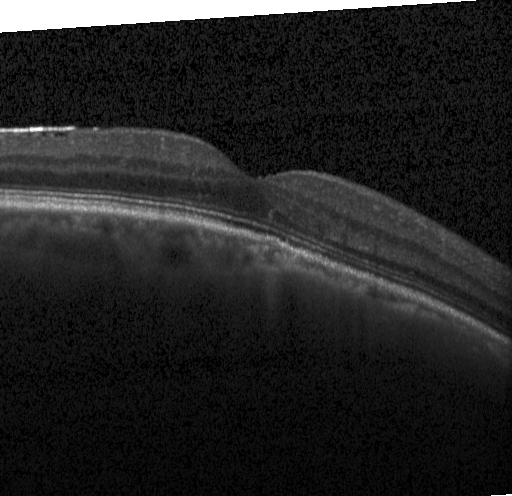

Impression: no evidence of CNV, DME, or drusen.